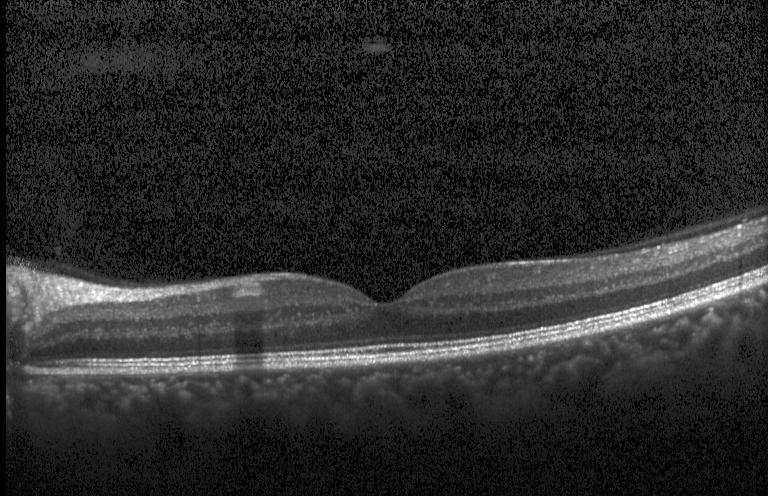 SD-OCT; optical coherence tomography scan
Assessment: no choroidal neovascularization, diabetic macular edema, or drusen.